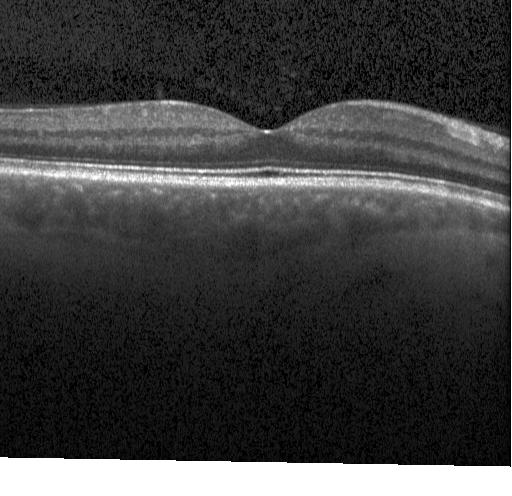 OCT B-scan — Finding: no choroidal neovascularization, diabetic macular edema, or drusen.